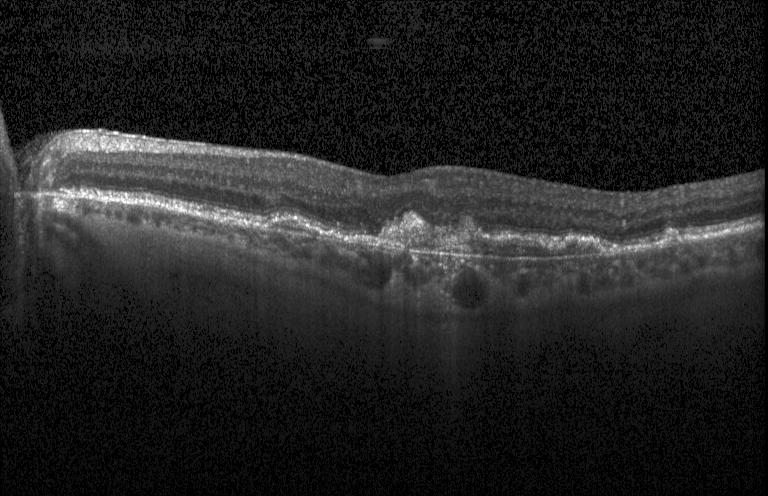

Finding: choroidal neovascularization.